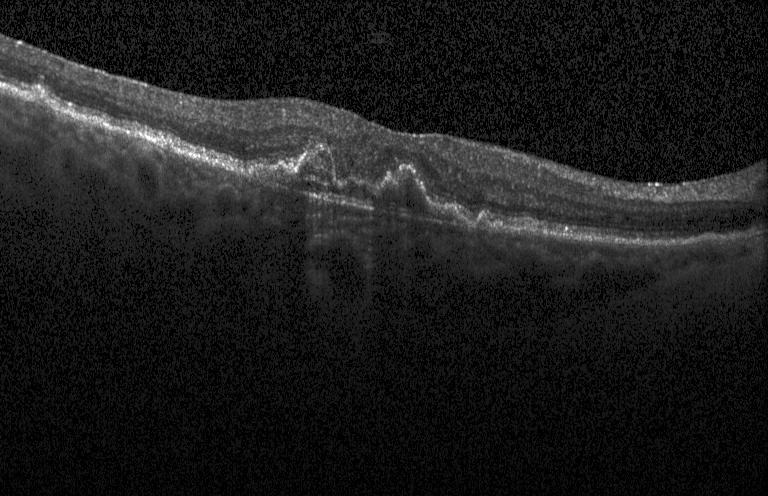 Retinal OCT cross-section · acquired on a Heidelberg Spectralis.
Diagnosis: choroidal neovascularization.